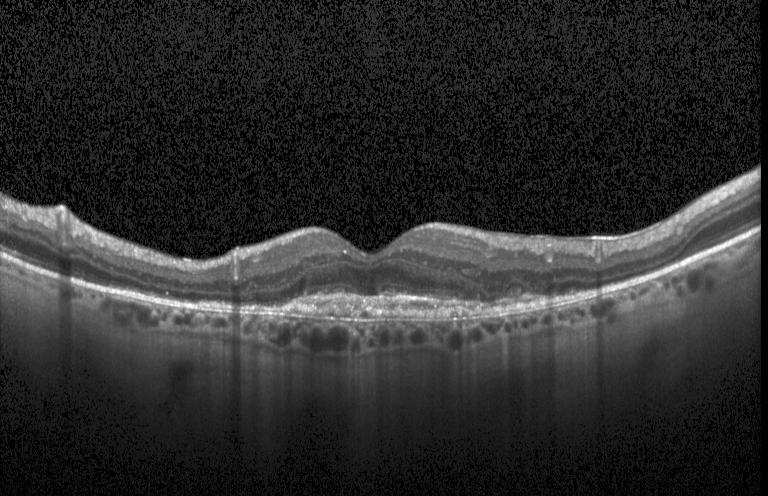
Instrument: Heidelberg Spectralis · horizontal scan through the fovea · SD-OCT · optical coherence tomography B-scan.
Diagnosis: choroidal neovascularization (CNV).